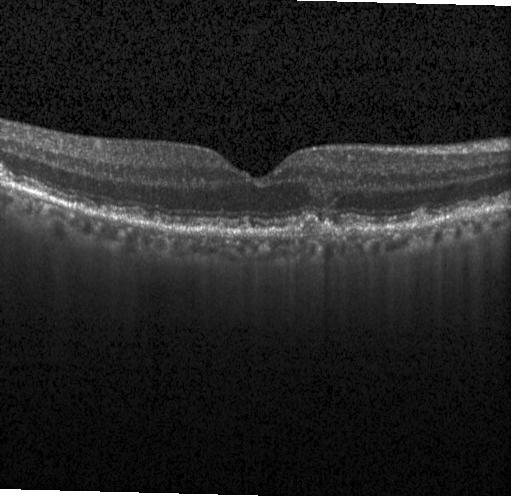
Optical coherence tomography scan; centered on the fovea.
Drusen.